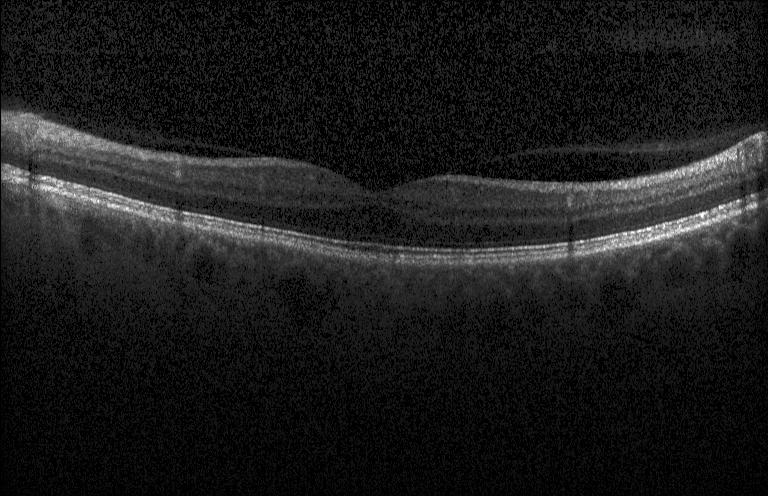
Optical coherence tomography scan. SD-OCT — Diagnosis: no CNV, no DME, and no drusen.